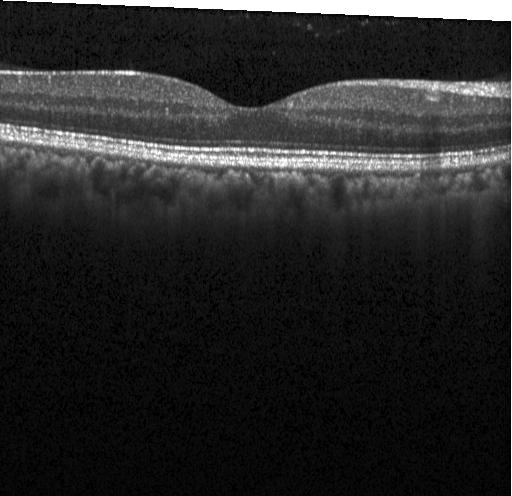 Finding: no choroidal neovascularization, no diabetic macular edema, and no drusen.